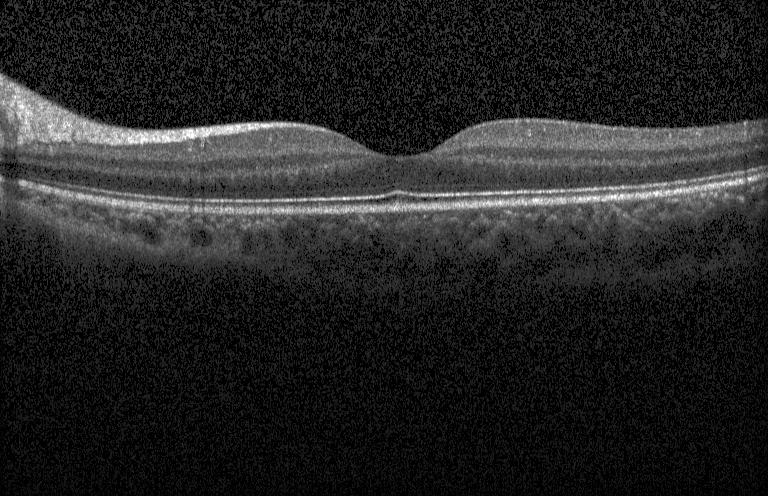
This B-scan demonstrates no choroidal neovascularization, no diabetic macular edema, and no drusen.